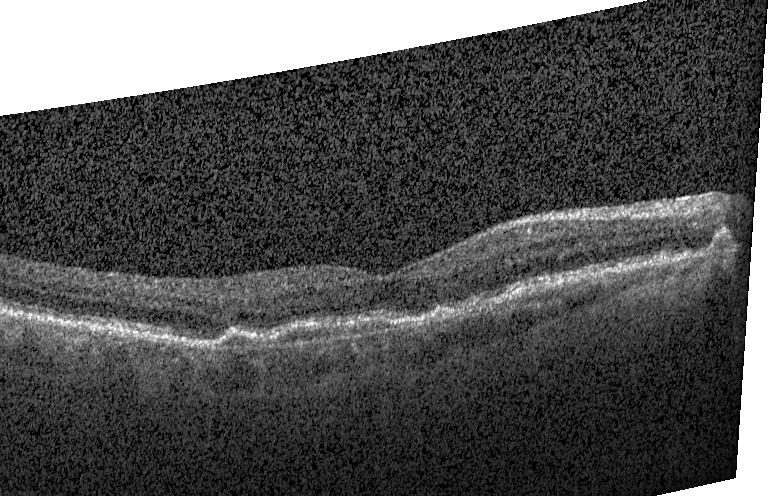 Optical coherence tomography scan, instrument: Heidelberg Spectralis
Dx: choroidal neovascularization.